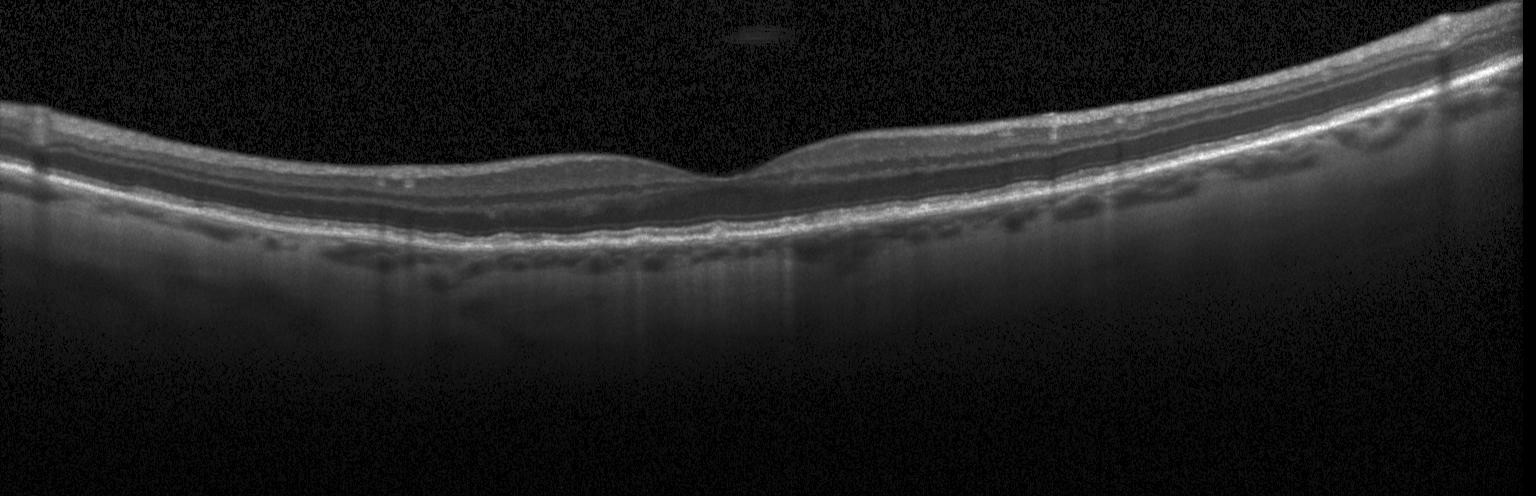 OCT B-scan
Impression: drusen.